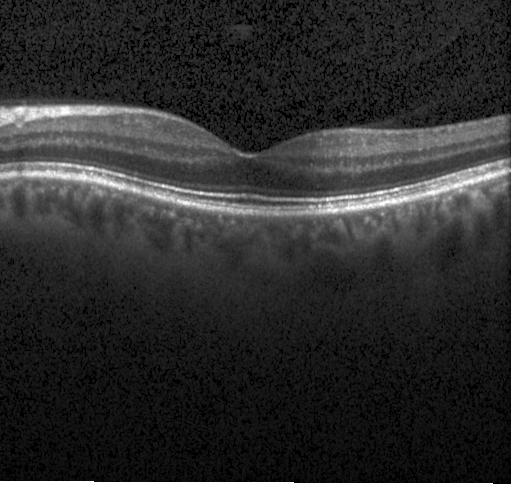 Retinal OCT B-scan; acquired on a Heidelberg Spectralis; horizontal scan through the fovea
Finding: no choroidal neovascularization, diabetic macular edema, or drusen.